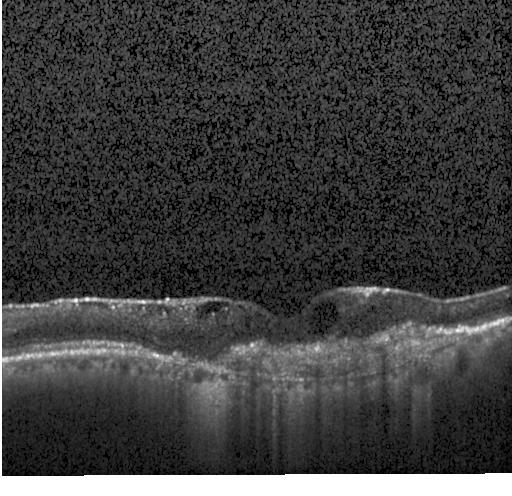

Retinal OCT cross-section. Impression: choroidal neovascularization (CNV).